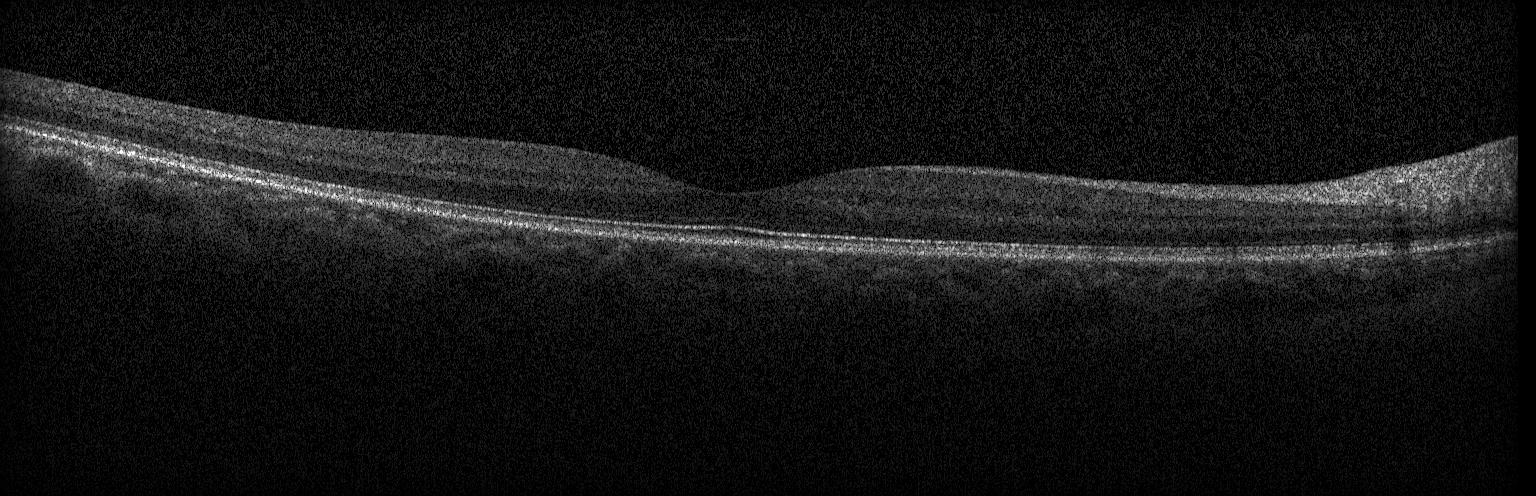

Retinal OCT cross-section. Heidelberg Spectralis OCT system.
No CNV, DME, or drusen.